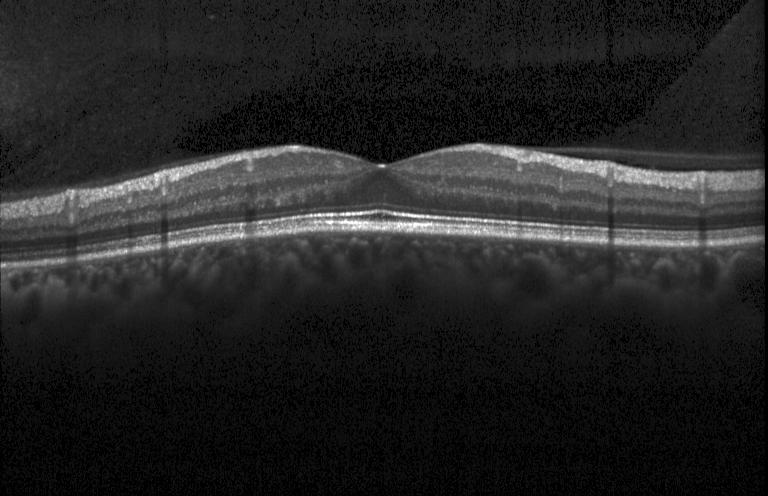 Retinal OCT B-scan — This B-scan demonstrates no choroidal neovascularization, diabetic macular edema, or drusen.